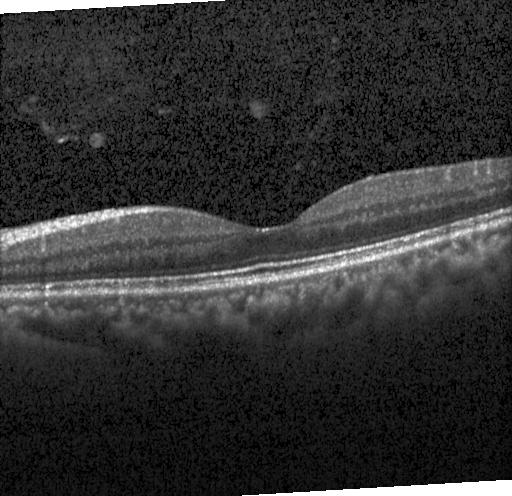

OCT B-scan.
Assessment: no choroidal neovascularization, diabetic macular edema, or drusen.